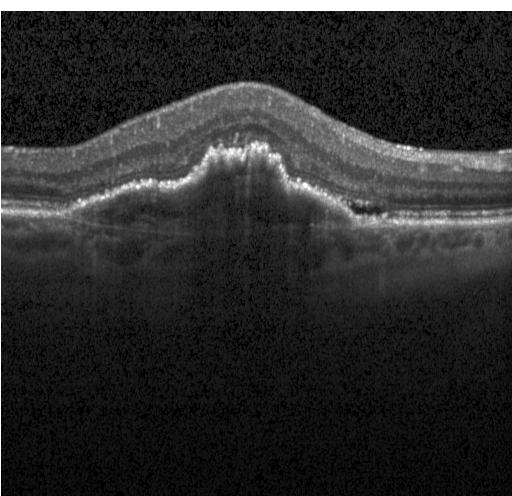

SD-OCT, macular scan, acquired on a Heidelberg Spectralis, retinal OCT B-scan. Impression: a choroidal neovascular membrane.